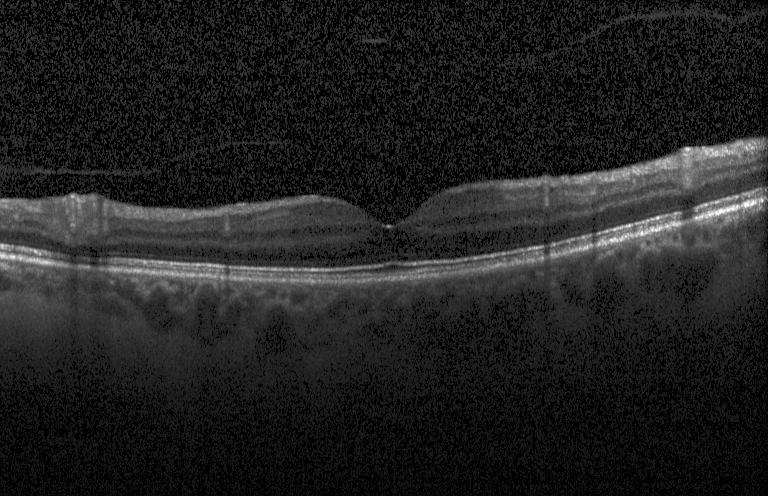

This B-scan demonstrates no evidence of CNV, DME, or drusen.